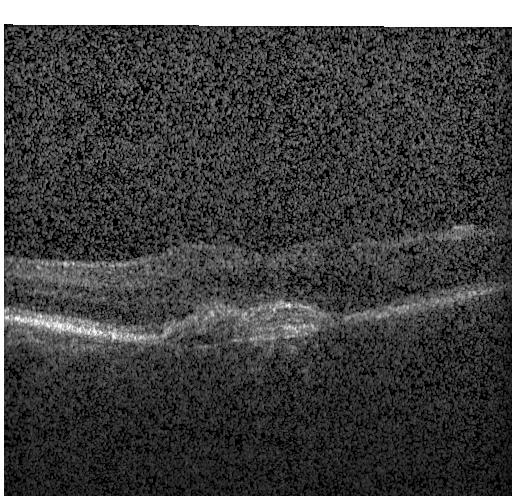
OCT B-scan showing choroidal neovascularization.